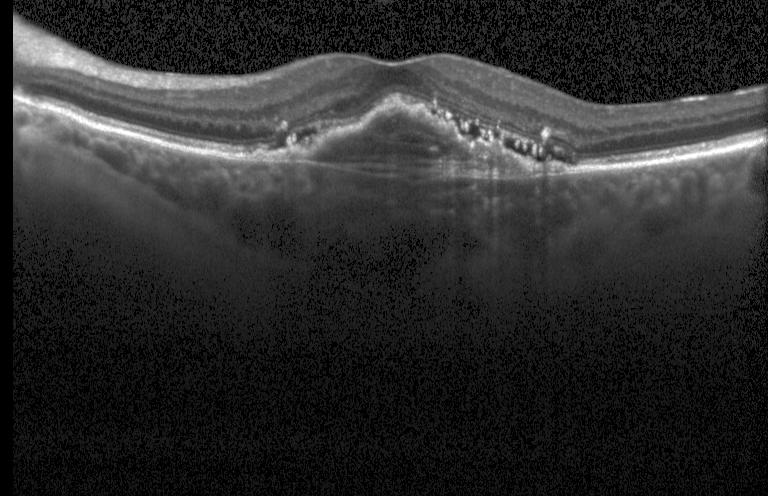
Retinal OCT cross-section. This B-scan demonstrates a choroidal neovascular membrane.